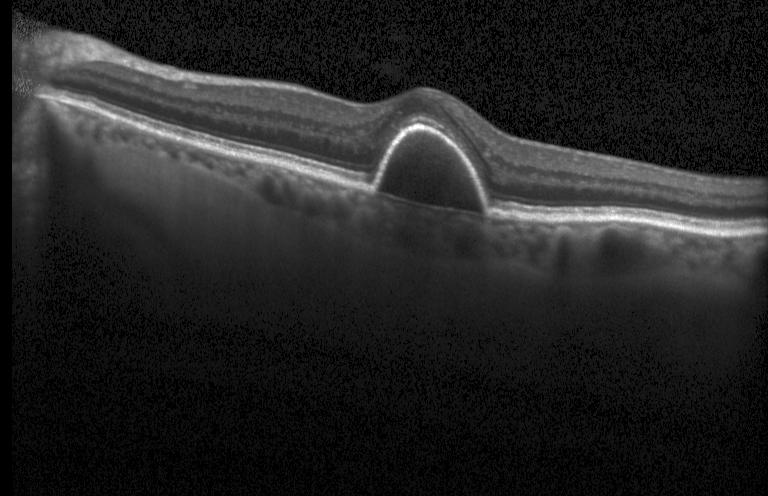

Optical coherence tomography B-scan — Finding: a choroidal neovascular membrane.